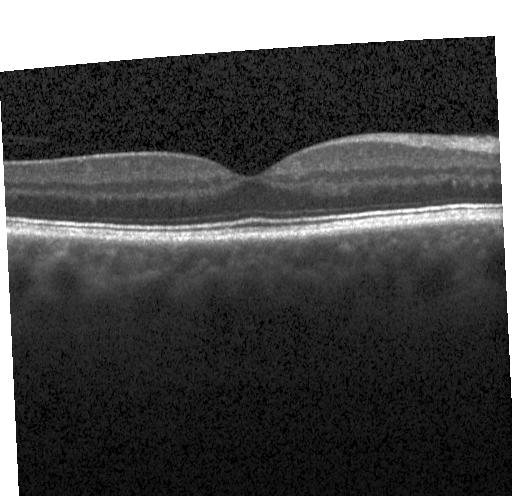 Heidelberg Spectralis OCT system · spectral-domain optical coherence tomography · retinal OCT B-scan.
Impression: neither choroidal neovascularization, diabetic macular edema, nor drusen.